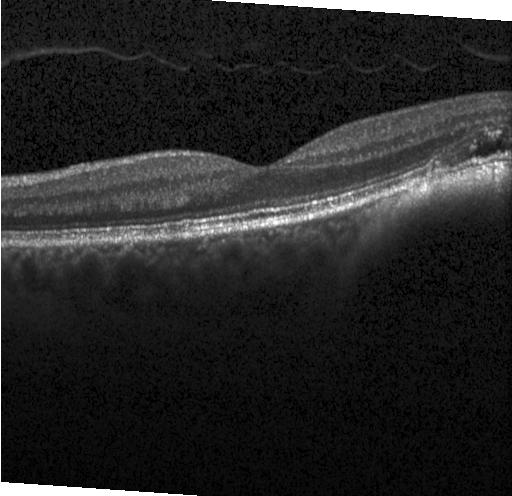
Impression: choroidal neovascularization (CNV).